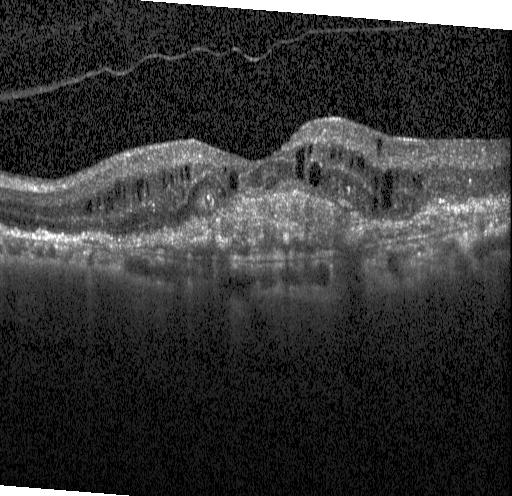
Dx: choroidal neovascularization (CNV).